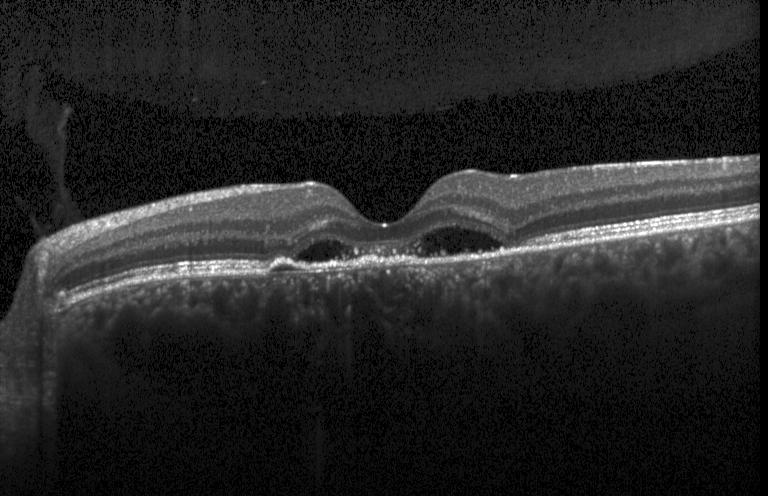 Optical coherence tomography B-scan. Assessment: choroidal neovascularization (CNV).